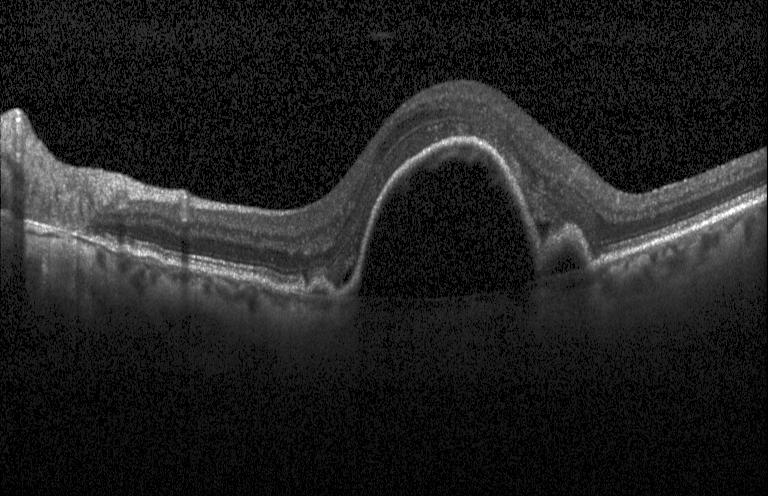 Assessment: choroidal neovascularization (CNV).